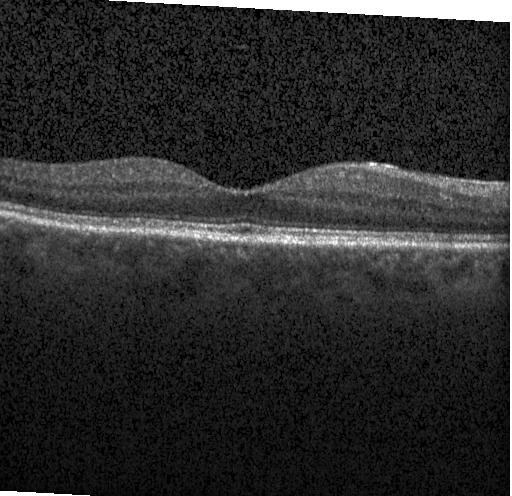 OCT line scan — Macular OCT: no choroidal neovascularization, no diabetic macular edema, and no drusen.